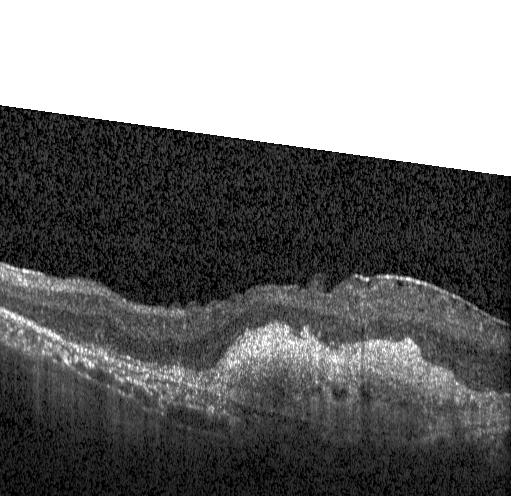 The scan shows a choroidal neovascular membrane.